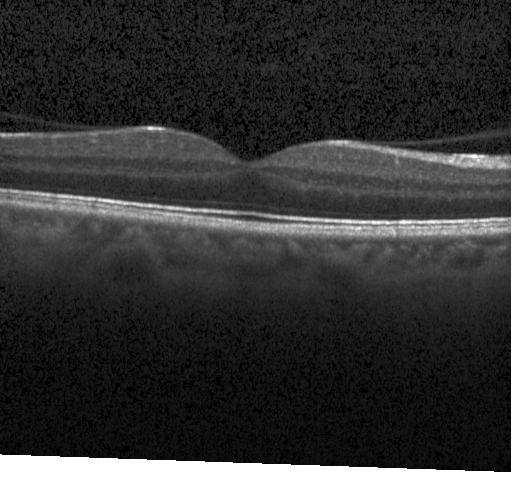 Impression: no choroidal neovascularization, no diabetic macular edema, and no drusen.